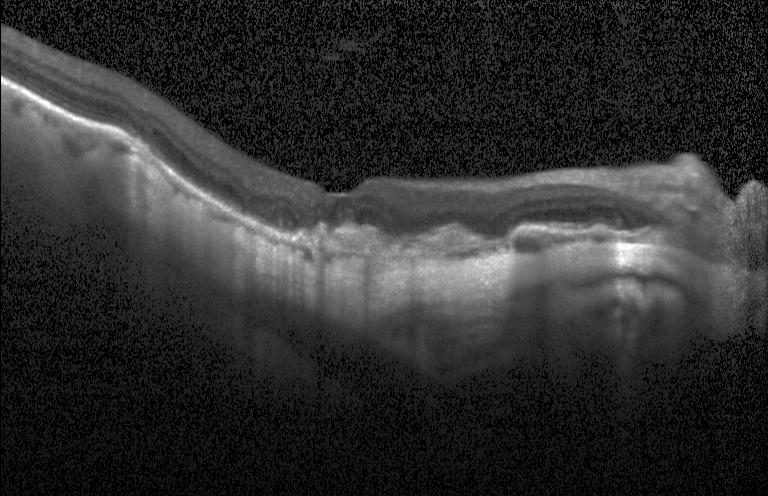
Retinal OCT B-scan
Macular OCT: a choroidal neovascular membrane.